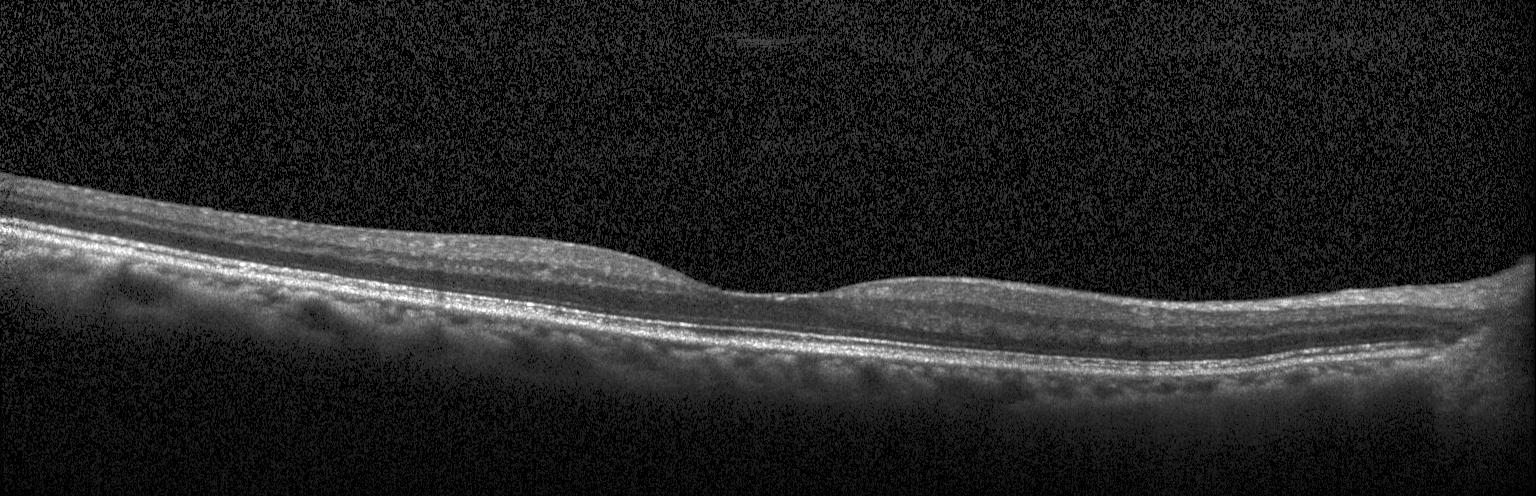

Retinal OCT cross-section. Impression: no evidence of choroidal neovascularization, diabetic macular edema, or drusen.